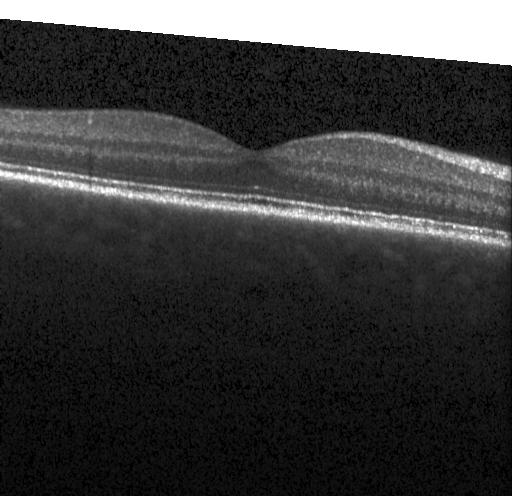 Optical coherence tomography scan, Heidelberg Spectralis OCT system. This B-scan demonstrates neither CNV, DME, nor drusen.